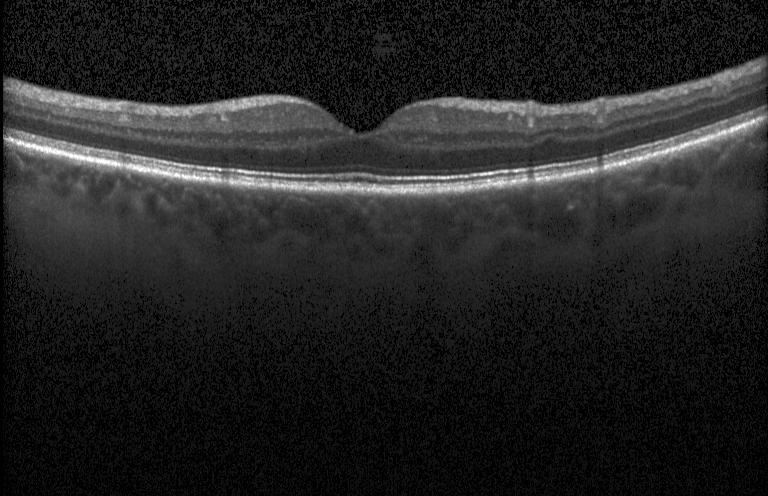

Assessment: neither CNV, DME, nor drusen.